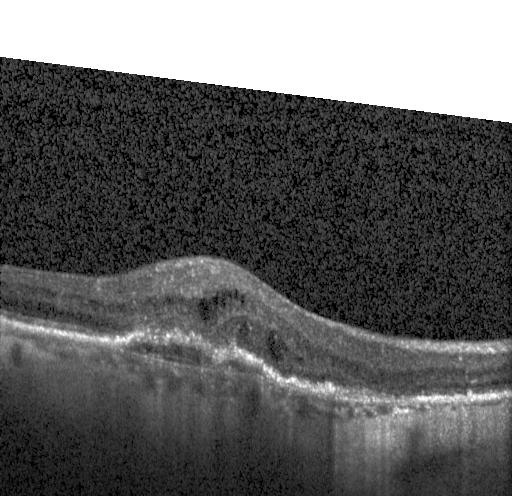 Heidelberg Spectralis OCT system · centered on the fovea · spectral-domain optical coherence tomography · OCT line scan.
Impression: a choroidal neovascular membrane.